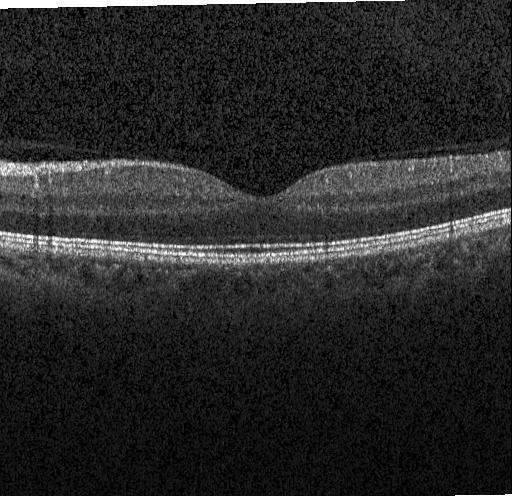 Horizontal scan through the fovea; optical coherence tomography scan. Impression: no choroidal neovascularization, diabetic macular edema, or drusen.